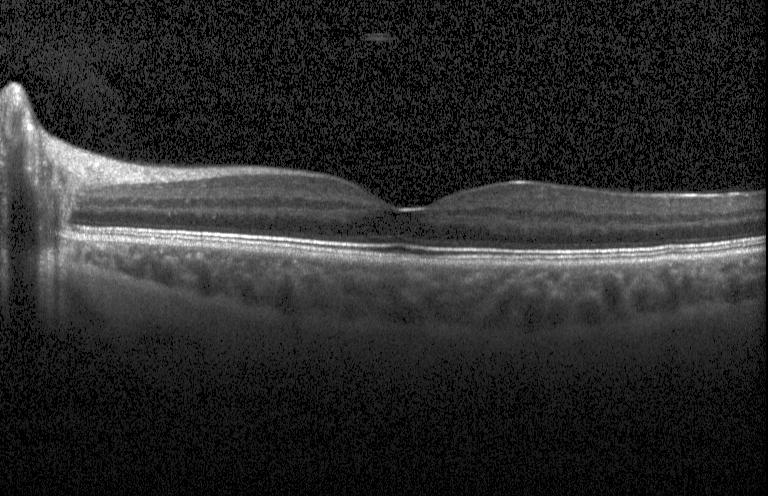
Finding: no evidence of CNV, DME, or drusen.